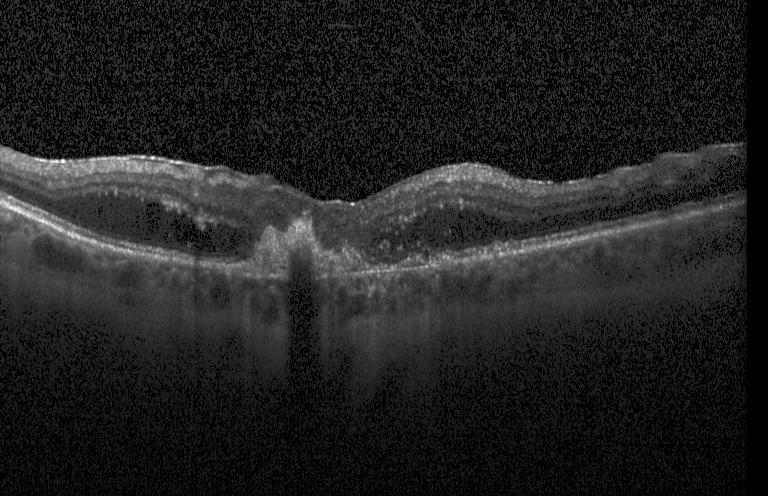 Finding: a choroidal neovascular membrane.